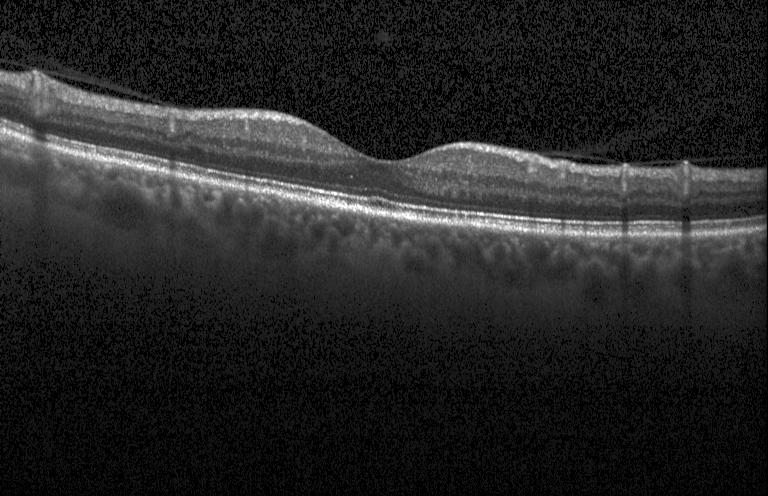

Retinal OCT B-scan, spectral-domain optical coherence tomography, through the macula, Heidelberg Spectralis
Diagnosis: no CNV, DME, or drusen.